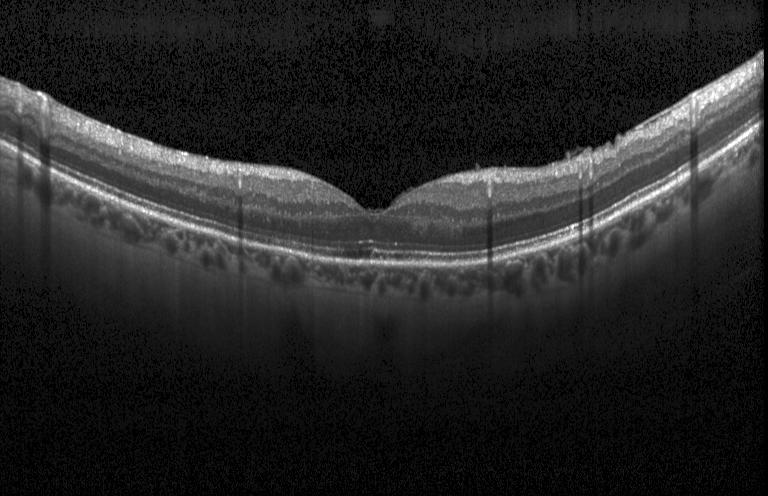

OCT B-scan — Impression: neither choroidal neovascularization, diabetic macular edema, nor drusen.